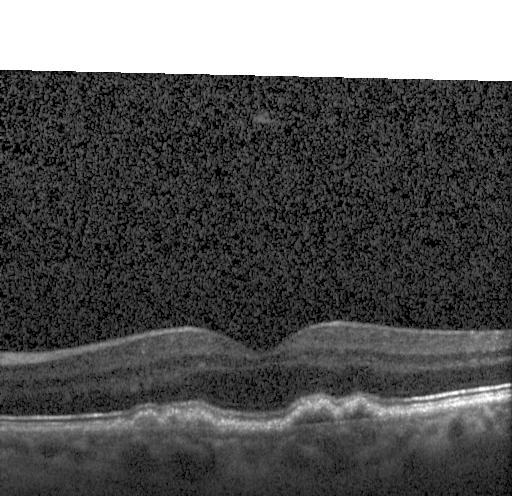
Instrument: Heidelberg Spectralis; optical coherence tomography scan; spectral-domain optical coherence tomography; through the macula
Dx: multiple drusen.